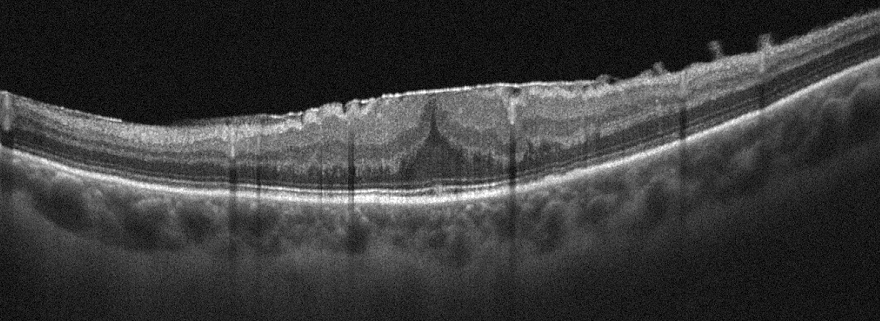
Retinal OCT B-scan.
Assessment: epiretinal membrane.